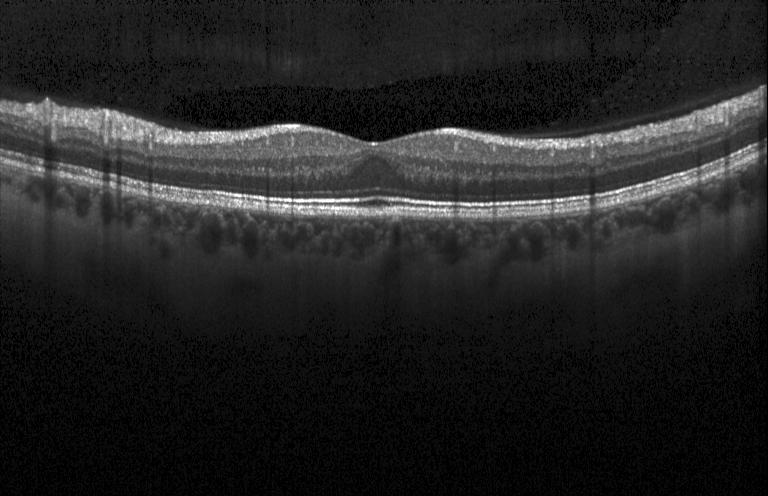 SD-OCT · OCT B-scan · instrument: Heidelberg Spectralis · fovea-centered — Assessment: no CNV, DME, or drusen.